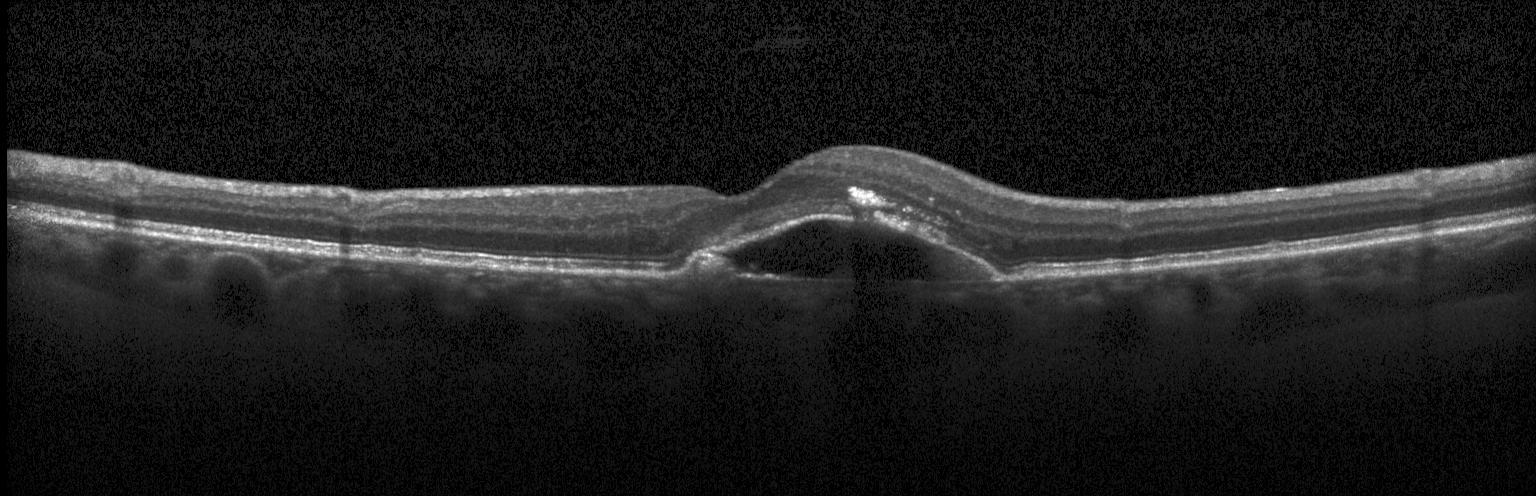

Instrument: Heidelberg Spectralis; OCT line scan. Impression: choroidal neovascularization.